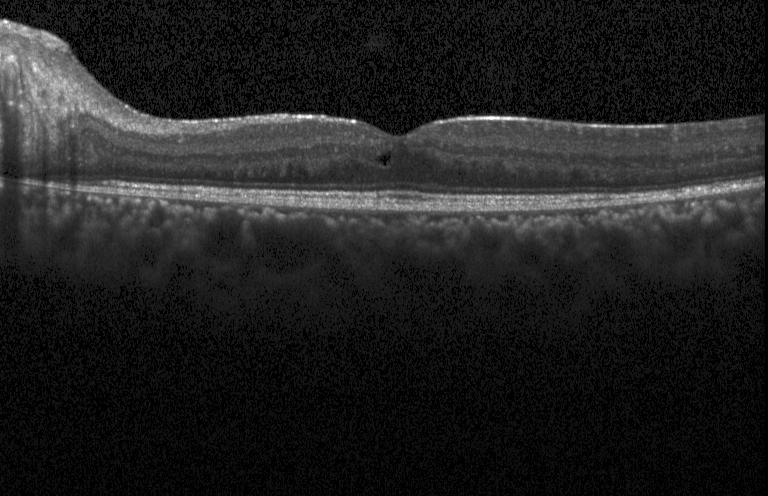

OCT line scan
Finding: diabetic macular edema.